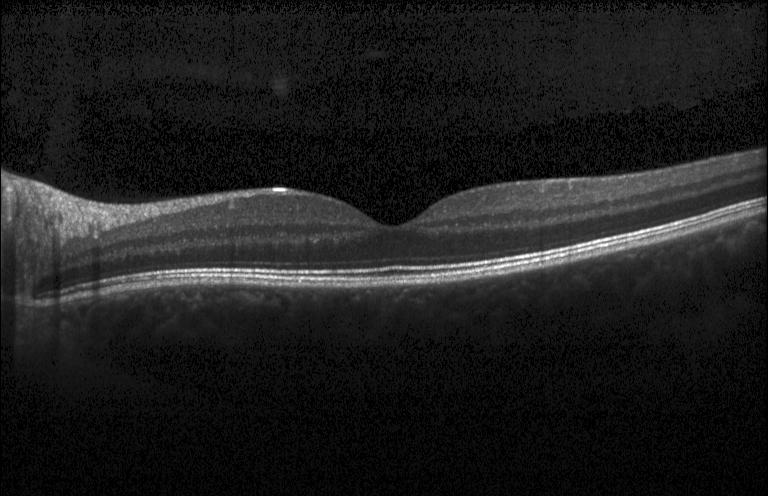 Spectral-domain optical coherence tomography; optical coherence tomography B-scan; Heidelberg Spectralis; through the macula. No CNV, no DME, and no drusen.